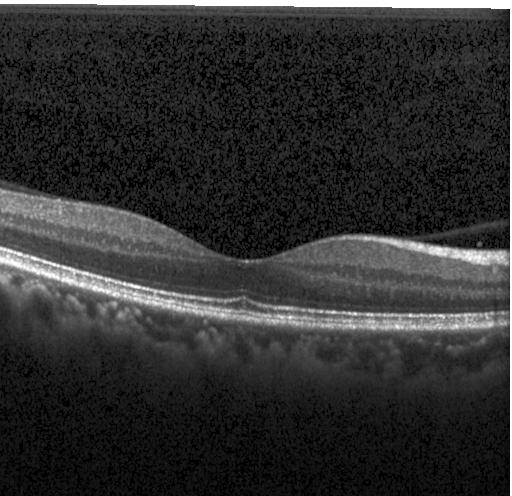
Retinal OCT cross-section. The scan shows no evidence of choroidal neovascularization, diabetic macular edema, or drusen.